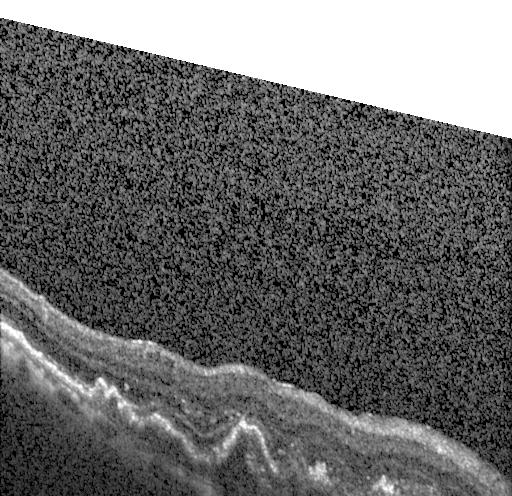

Optical coherence tomography B-scan; spectral-domain optical coherence tomography — Impression: a choroidal neovascular membrane.